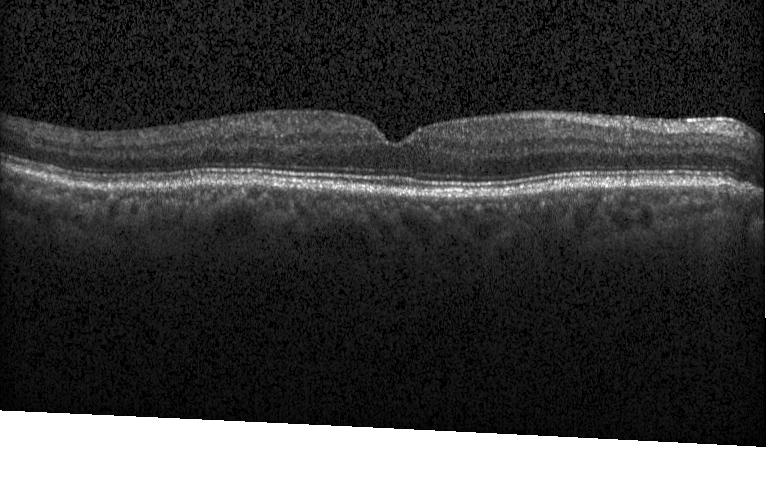
The scan shows no CNV, DME, or drusen.